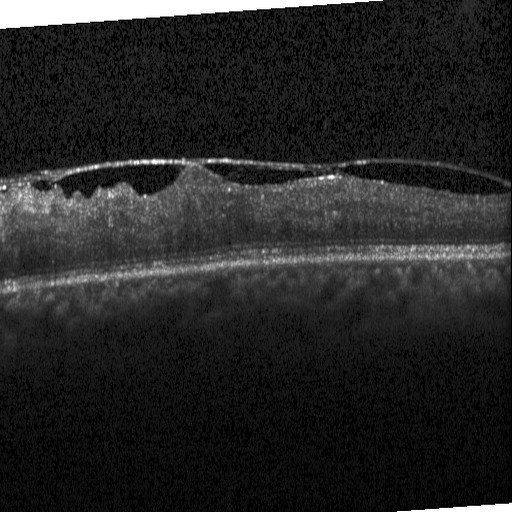 OCT B-scan. Dx: diabetic macular edema.